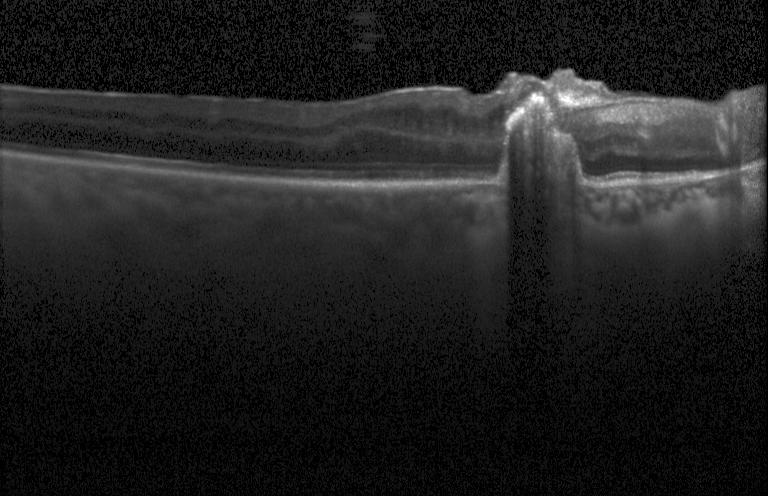 Macular OCT demonstrating a choroidal neovascular membrane.